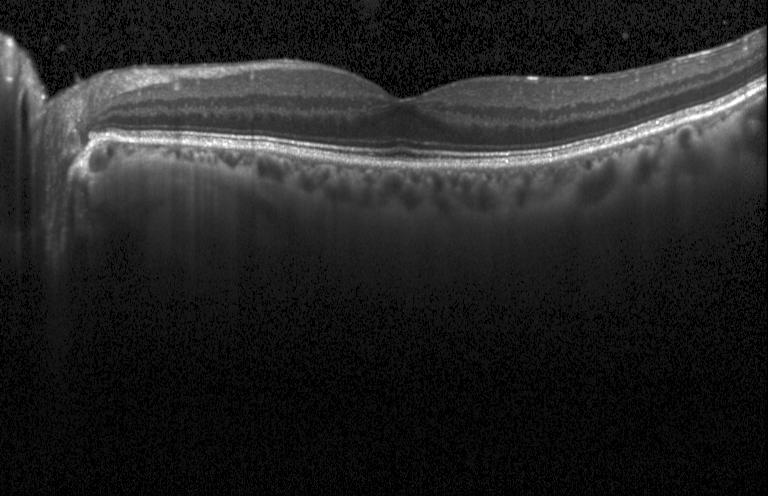 OCT finding: no evidence of choroidal neovascularization, diabetic macular edema, or drusen.